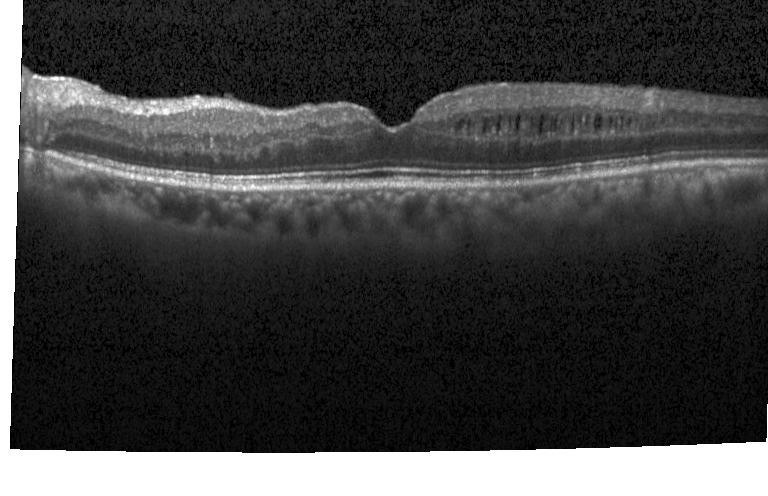
Optical coherence tomography scan · instrument: Heidelberg Spectralis
Finding: DME.